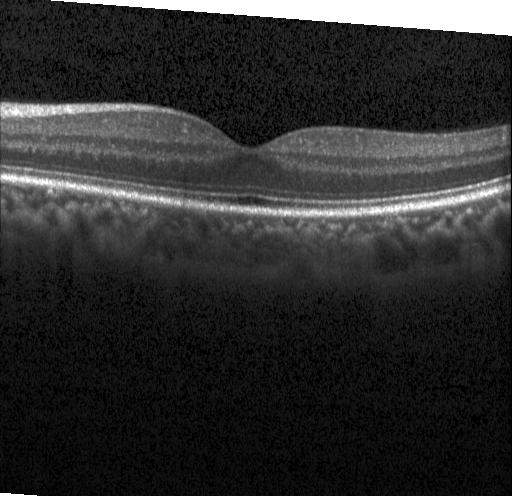 Spectral-domain OCT B-scan: no choroidal neovascularization, no diabetic macular edema, and no drusen.